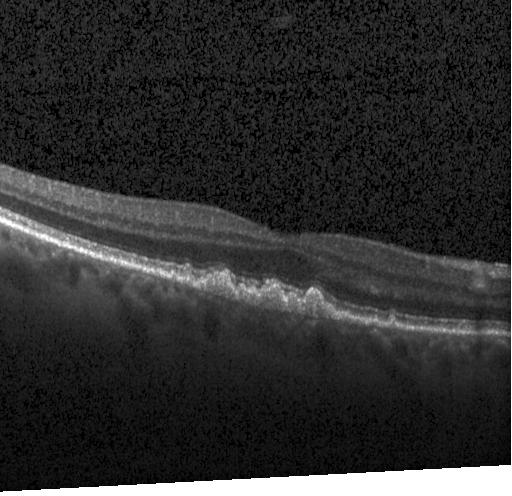
Retinal OCT cross-section
Diagnosis: sub-RPE drusenoid deposits.